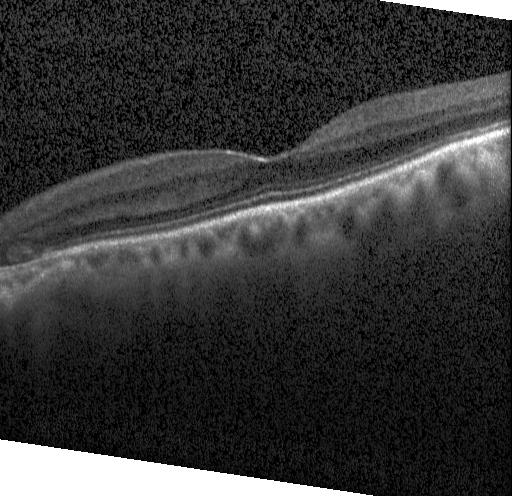 OCT line scan.
No choroidal neovascularization, diabetic macular edema, or drusen.